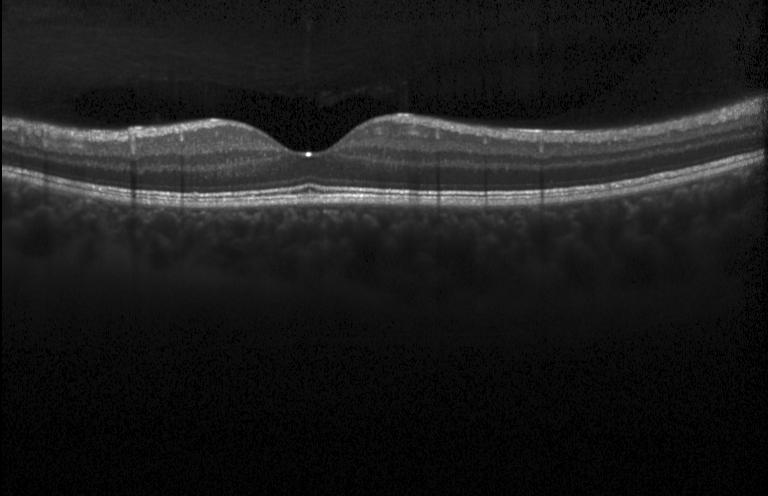

Spectral-domain optical coherence tomography, instrument: Heidelberg Spectralis, fovea-centered, retinal OCT B-scan. No evidence of choroidal neovascularization, diabetic macular edema, or drusen.